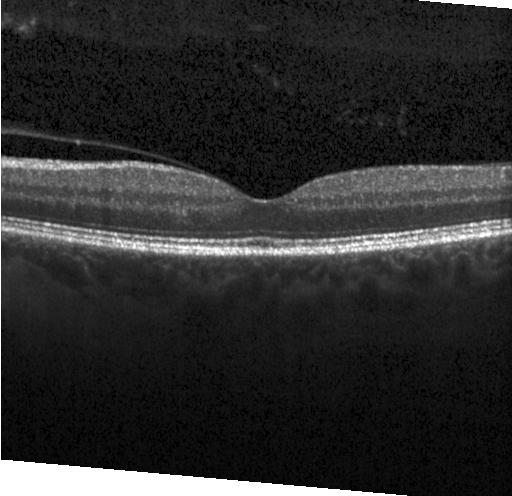 OCT finding: no choroidal neovascularization, diabetic macular edema, or drusen.